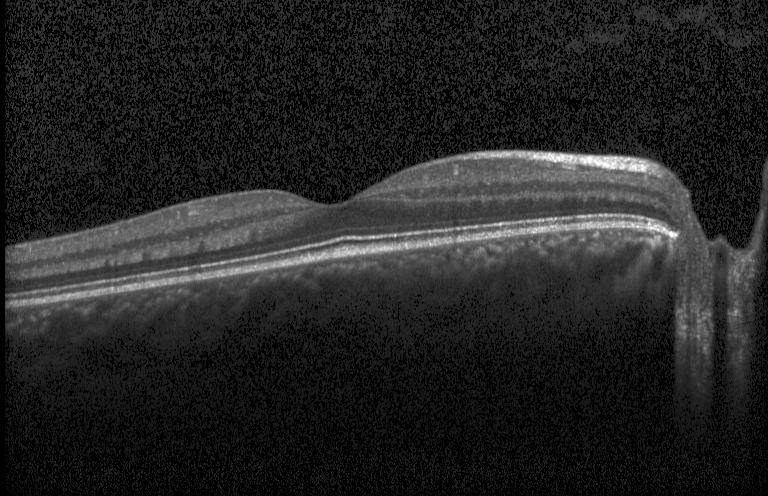 Spectral-domain OCT B-scan: no choroidal neovascularization, no diabetic macular edema, and no drusen.